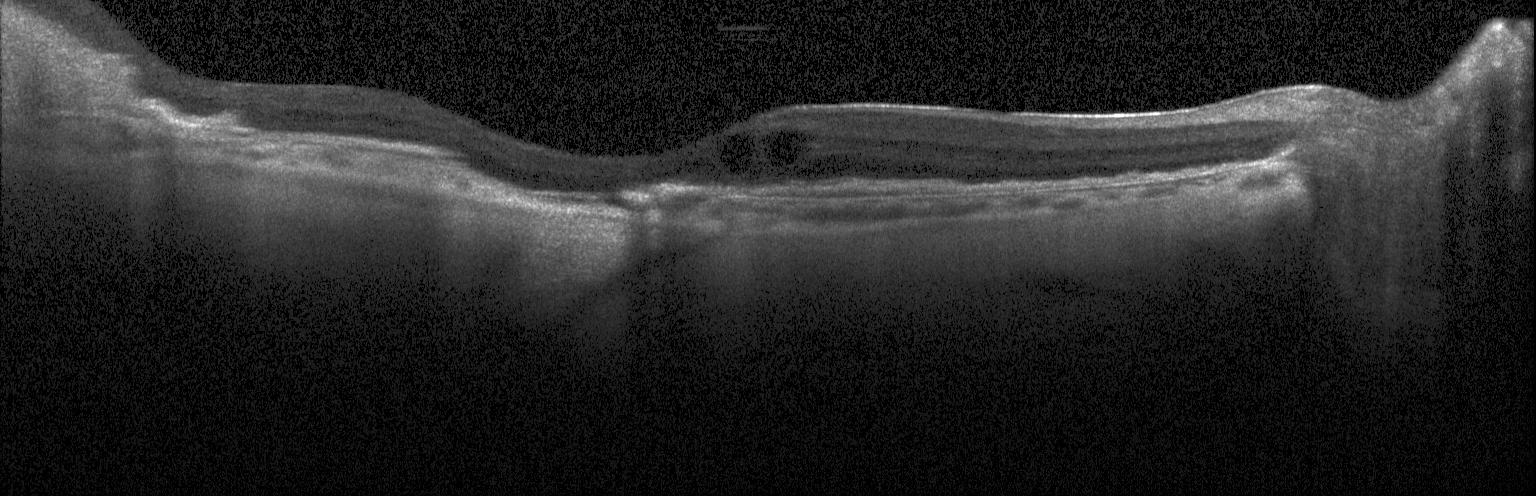

Diagnosis: choroidal neovascularization (CNV).